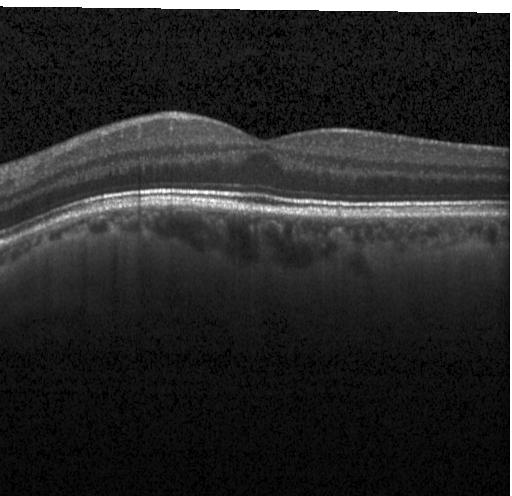
Optical coherence tomography B-scan — Assessment: neither CNV, DME, nor drusen.